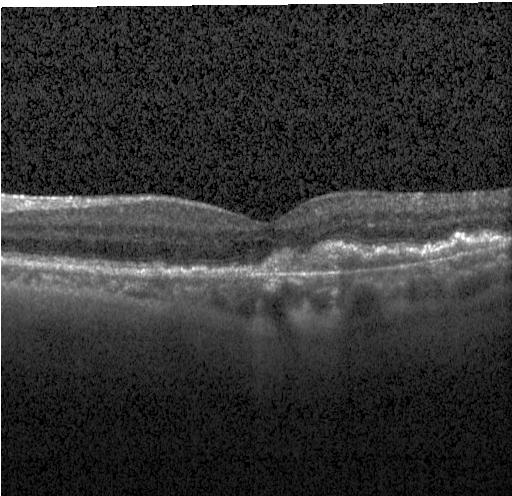 Through the macula · optical coherence tomography scan.
Choroidal neovascularization (CNV).